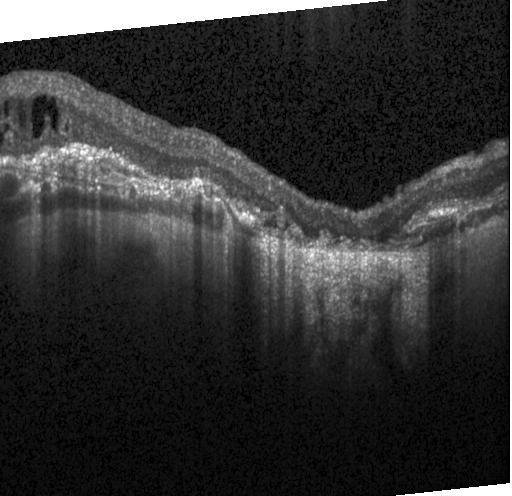
Diagnosis: CNV.